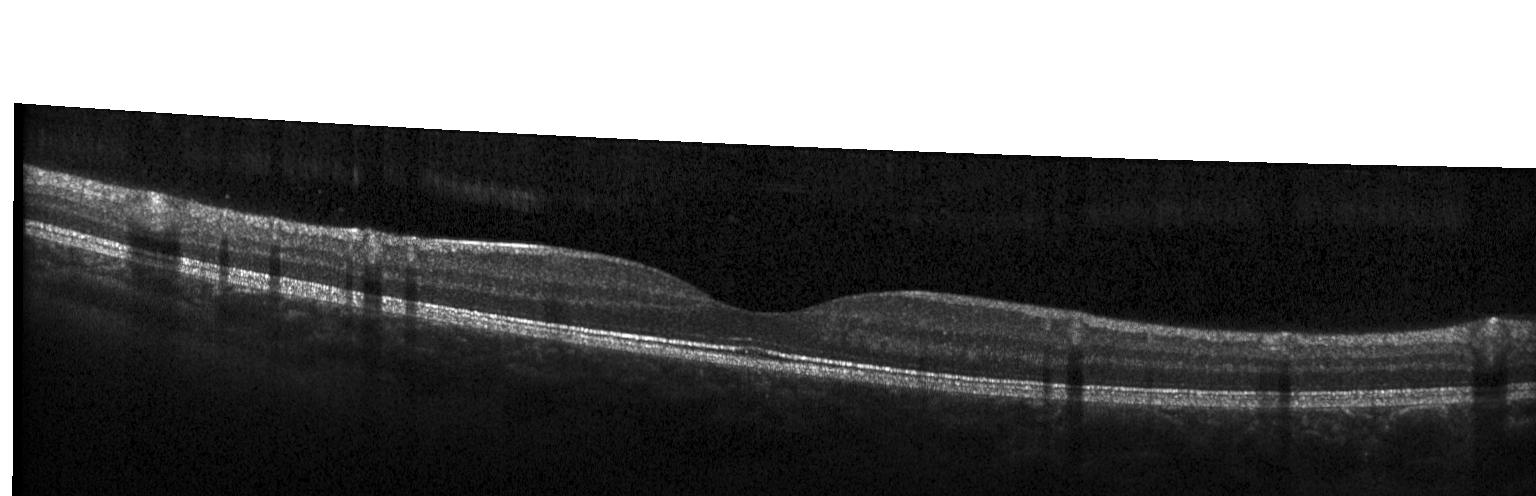
OCT B-scan. No choroidal neovascularization, no diabetic macular edema, and no drusen.